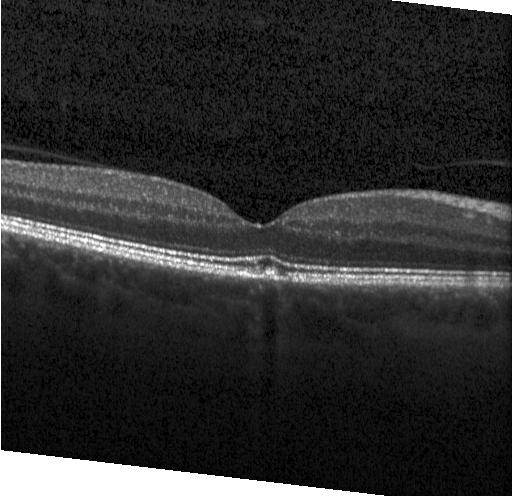 Impression: no CNV, DME, or drusen.